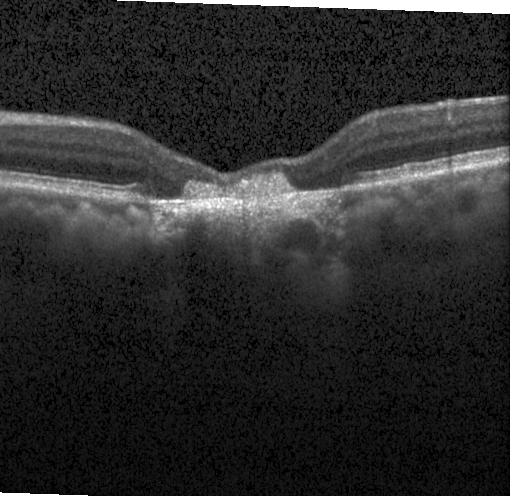
Optical coherence tomography B-scan · through the macula · spectral-domain OCT · instrument: Heidelberg Spectralis
A choroidal neovascular membrane.